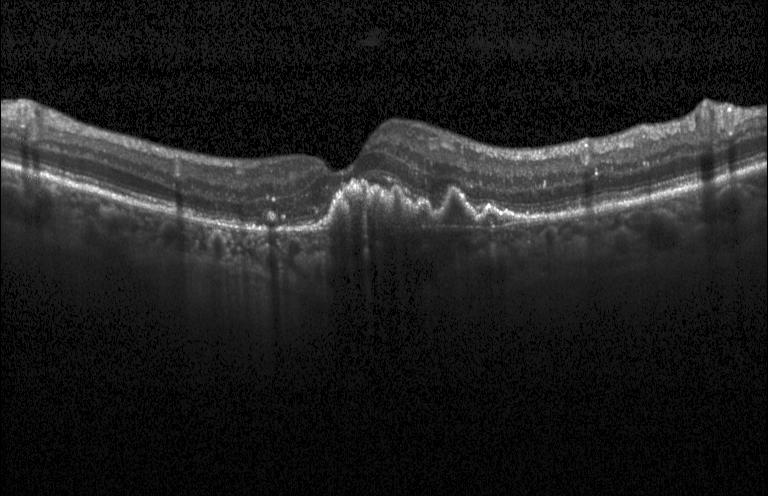 Retinal OCT B-scan · spectral-domain optical coherence tomography · horizontal scan through the fovea.
Diagnosis: CNV.